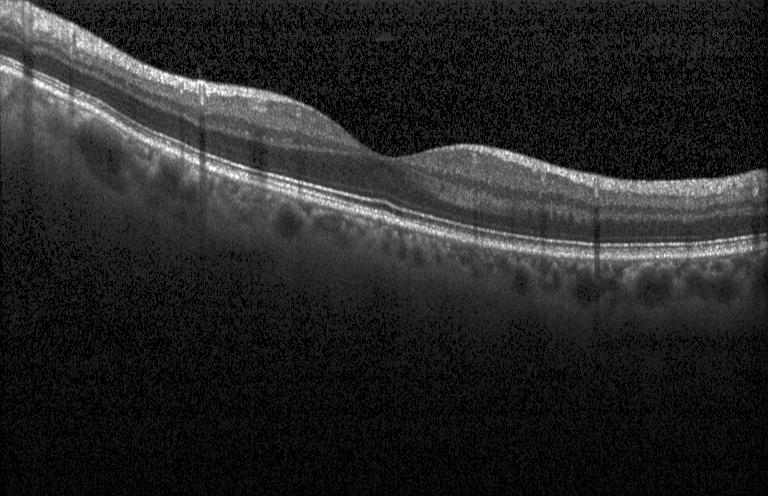

OCT finding: no choroidal neovascularization, no diabetic macular edema, and no drusen.